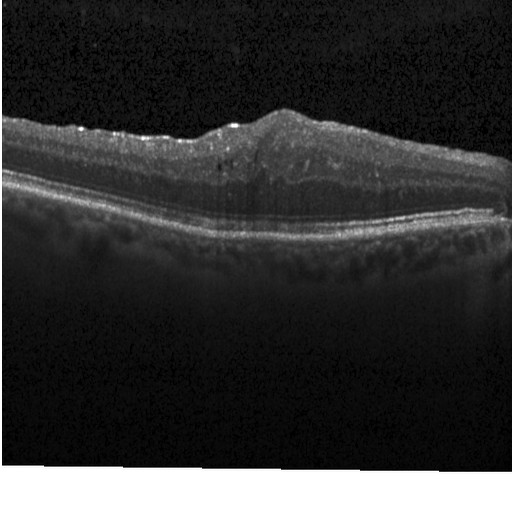
Impression: diabetic macular edema (DME).